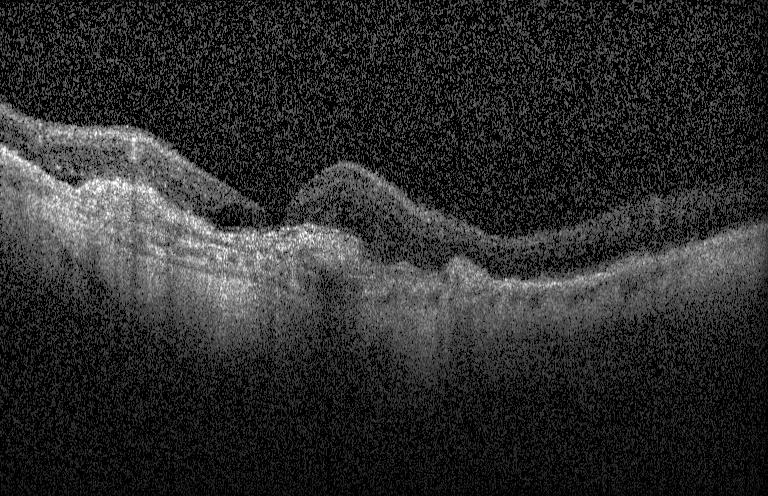

Spectral-domain OCT · acquired on a Heidelberg Spectralis · centered on the fovea · retinal OCT B-scan — Impression: choroidal neovascularization.